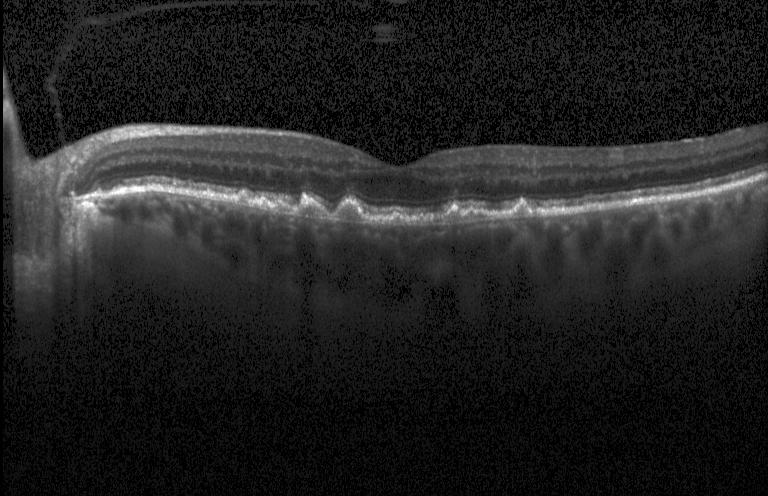 OCT B-scan showing drusen.